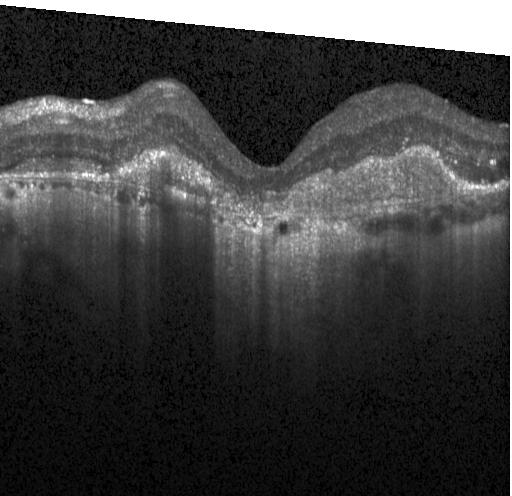
Macular OCT: choroidal neovascularization.